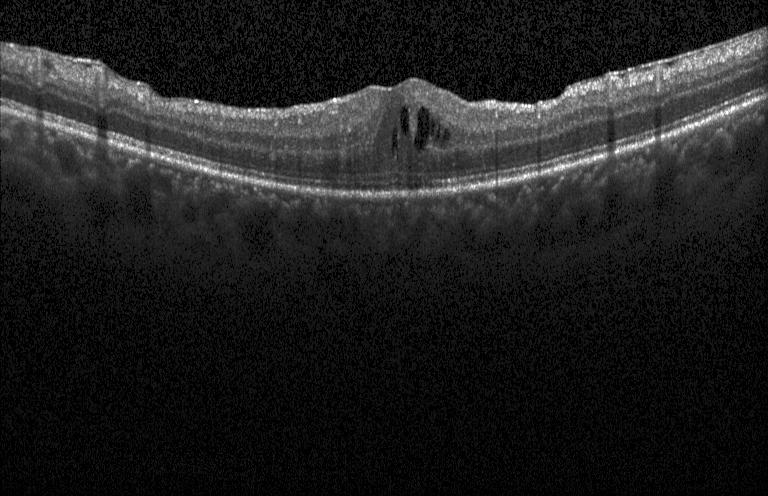

OCT B-scan showing DME.